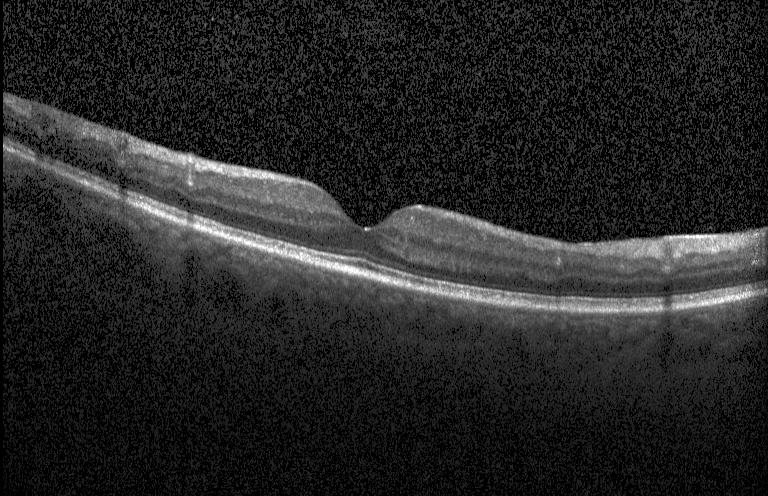 Finding: neither CNV, DME, nor drusen.